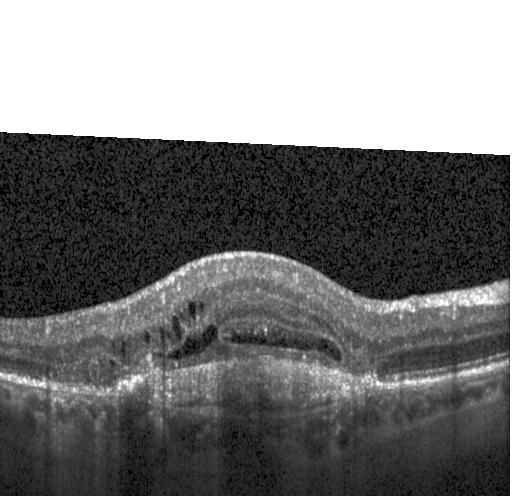
Spectral-domain optical coherence tomography; instrument: Heidelberg Spectralis; centered on the fovea; optical coherence tomography B-scan.
Impression: a choroidal neovascular membrane.